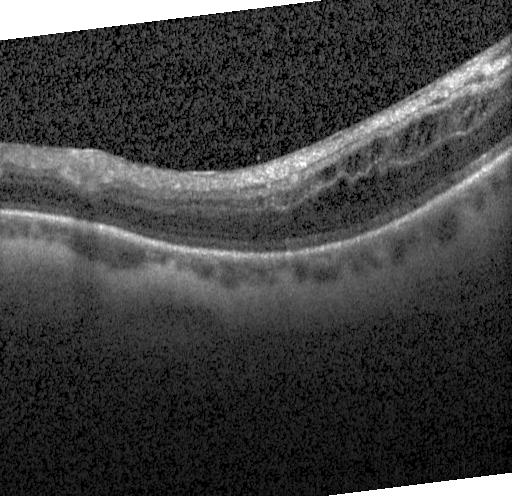
Finding: DME.